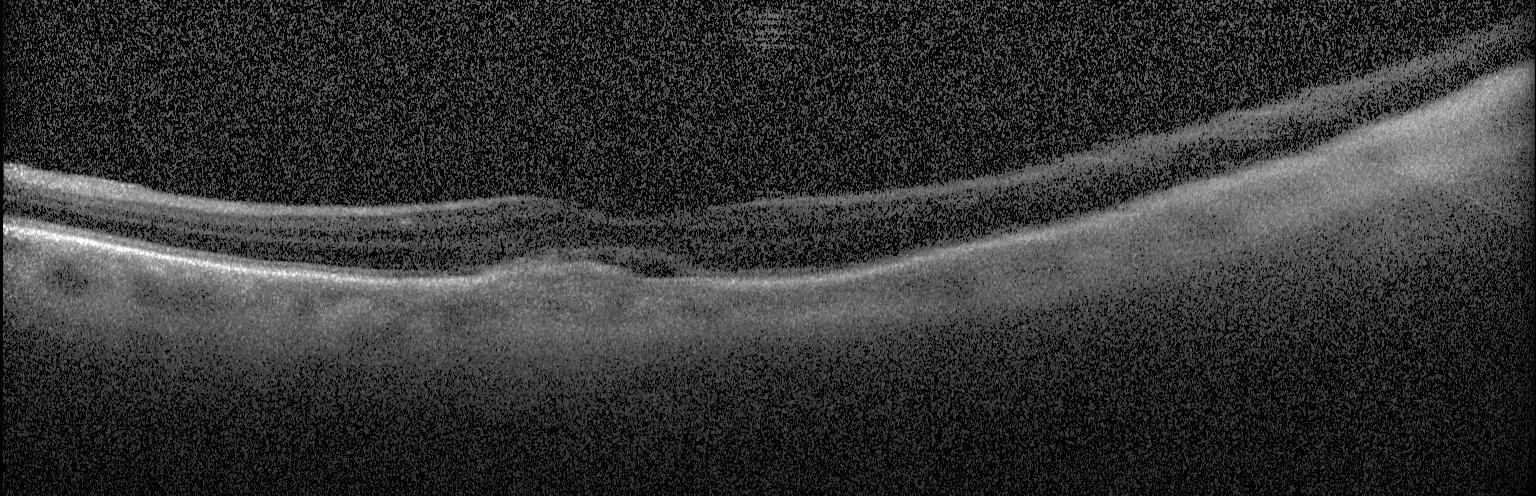

Macular scan; optical coherence tomography scan; spectral-domain optical coherence tomography. A choroidal neovascular membrane.